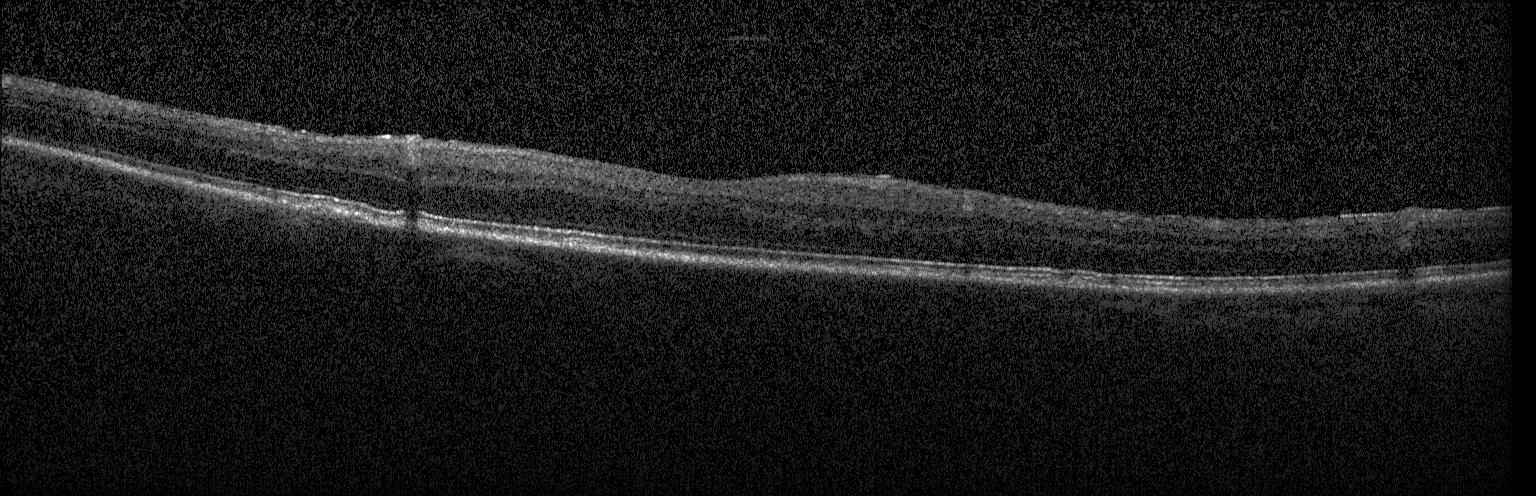

Macular OCT: neither choroidal neovascularization, diabetic macular edema, nor drusen.